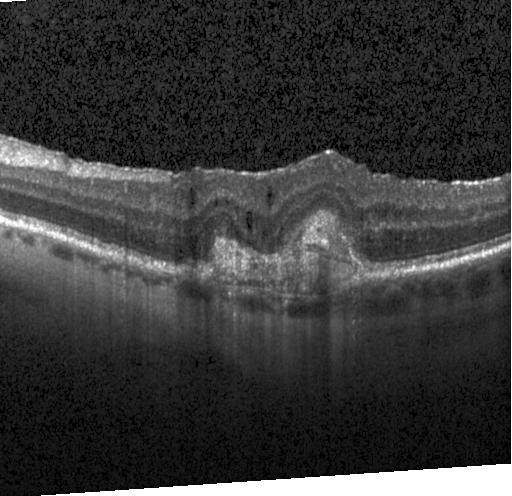
Retinal OCT B-scan. Horizontal scan through the fovea
Diagnosis: a choroidal neovascular membrane.